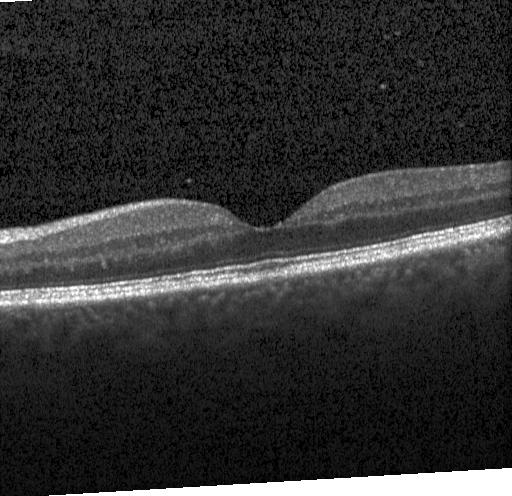 Centered on the fovea; retinal OCT cross-section; spectral-domain optical coherence tomography; acquired on a Heidelberg Spectralis — Diagnosis: no choroidal neovascularization, diabetic macular edema, or drusen.